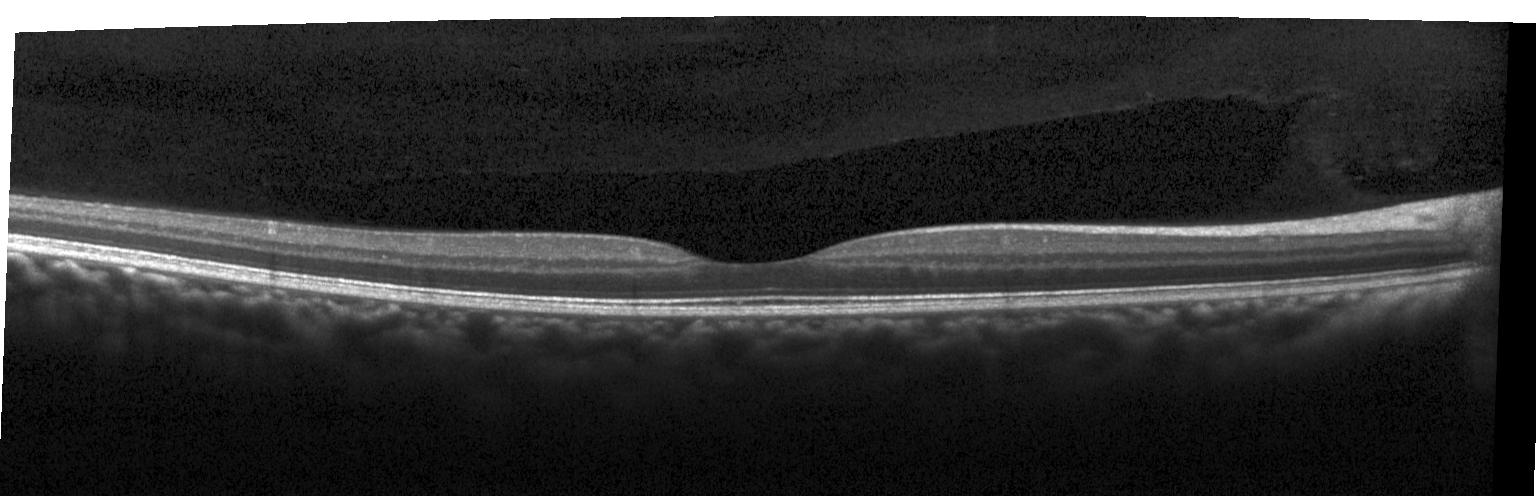 Retinal OCT cross-section
Finding: neither CNV, DME, nor drusen.